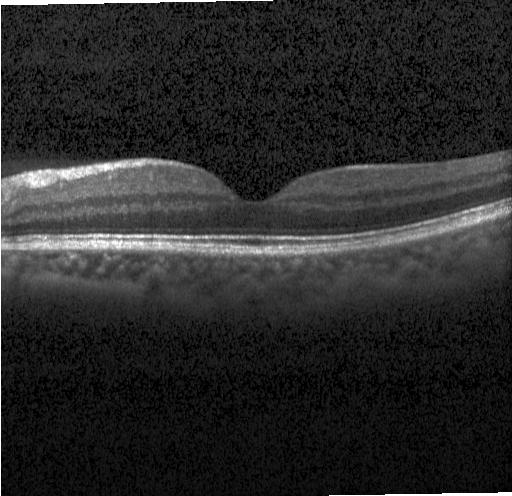
Centered on the fovea; Heidelberg Spectralis OCT system; spectral-domain OCT; retinal OCT cross-section — Diagnosis: no choroidal neovascularization, no diabetic macular edema, and no drusen.